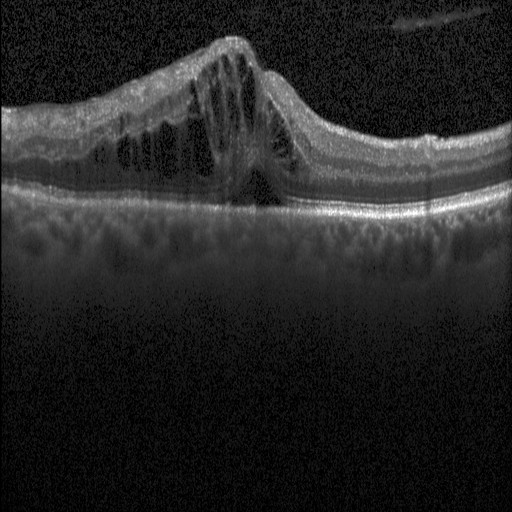

SD-OCT; horizontal scan through the fovea; optical coherence tomography scan
Impression: diabetic macular edema.